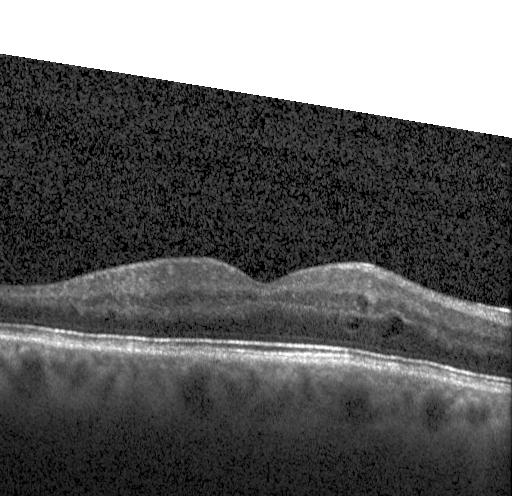
SD-OCT · retinal OCT B-scan · Heidelberg Spectralis OCT system — Finding: DME.